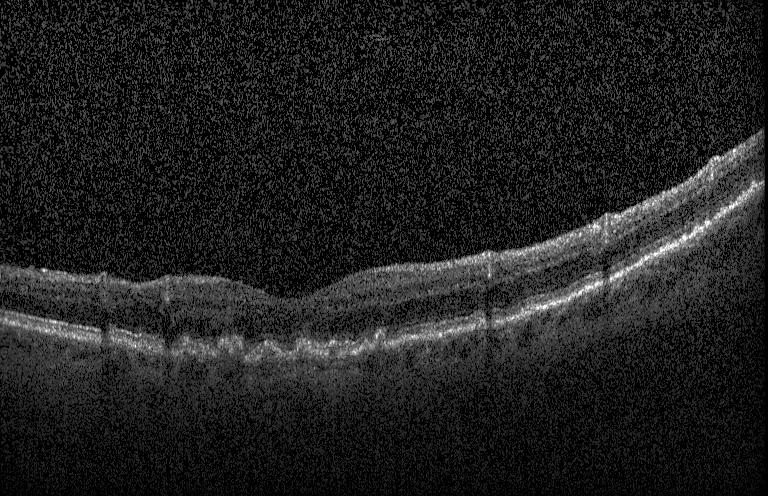

Diagnosis: multiple drusen.